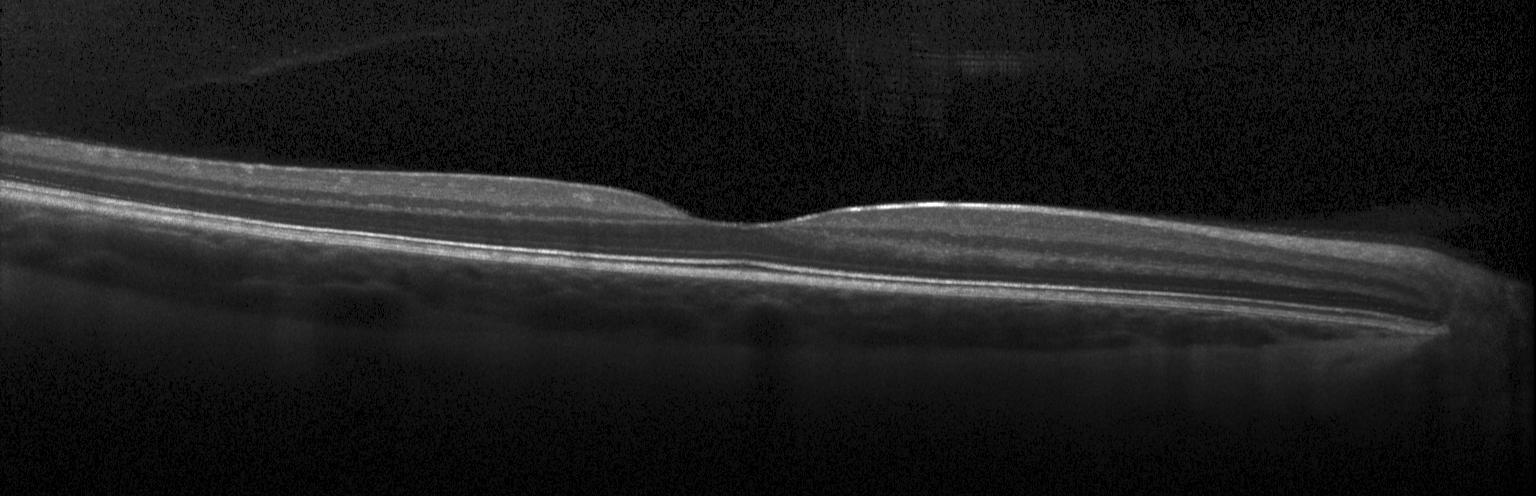

Retinal OCT cross-section — Impression: no CNV, DME, or drusen.